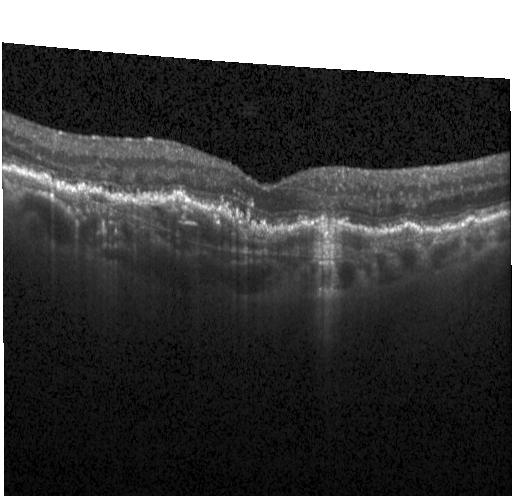

OCT B-scan showing choroidal neovascularization (CNV).